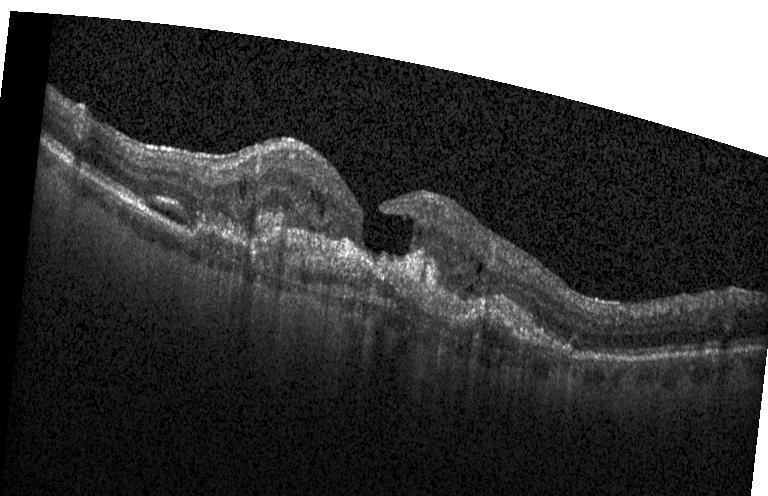

The scan shows a choroidal neovascular membrane.